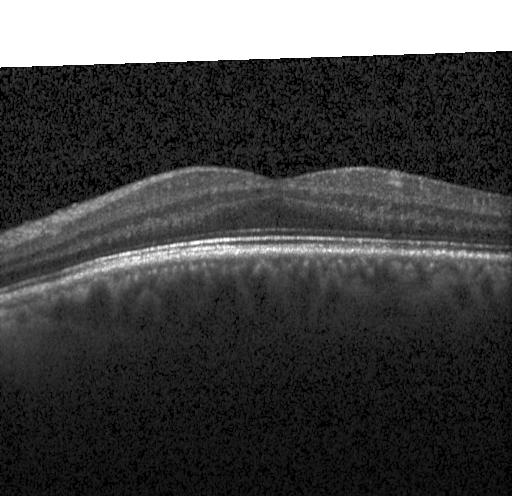
Macular scan. Optical coherence tomography scan. Spectral-domain OCT
Assessment: no CNV, no DME, and no drusen.